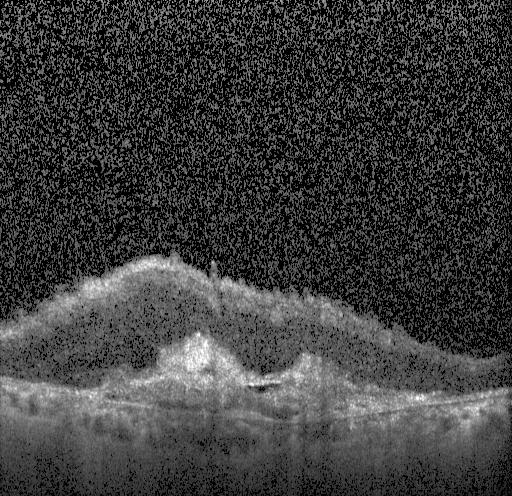 Retinal OCT cross-section showing choroidal neovascularization.